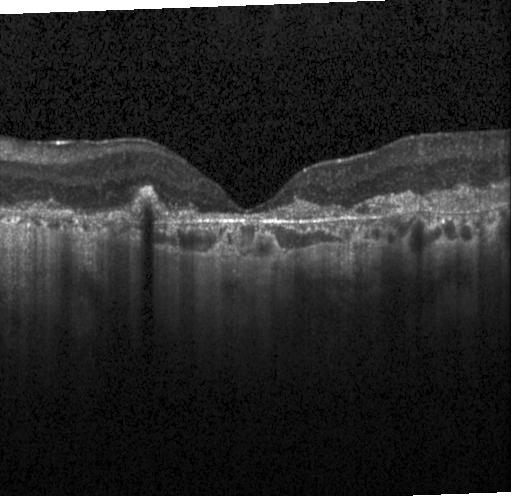

Assessment: a choroidal neovascular membrane.